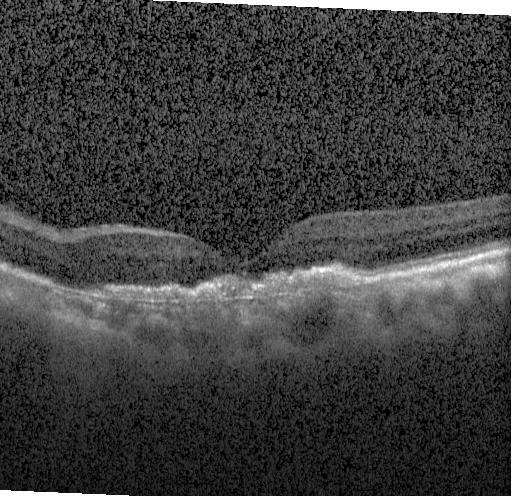 OCT line scan
Diagnosis: choroidal neovascularization (CNV).